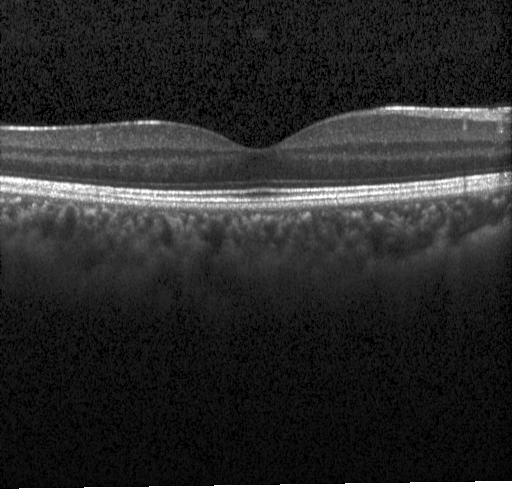

Retinal OCT cross-section showing no CNV, DME, or drusen.